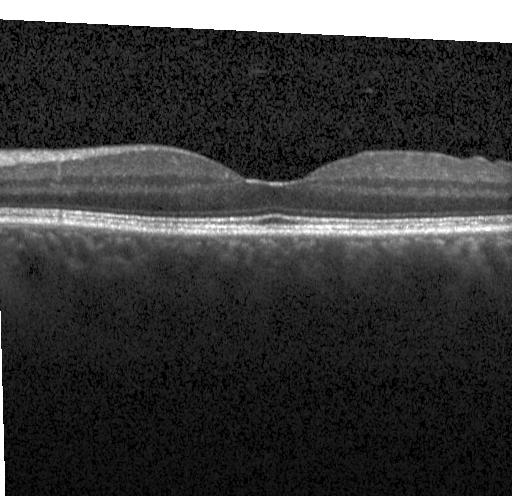
Optical coherence tomography scan; acquired on a Heidelberg Spectralis; horizontal scan through the fovea; spectral-domain optical coherence tomography — This B-scan demonstrates no CNV, DME, or drusen.